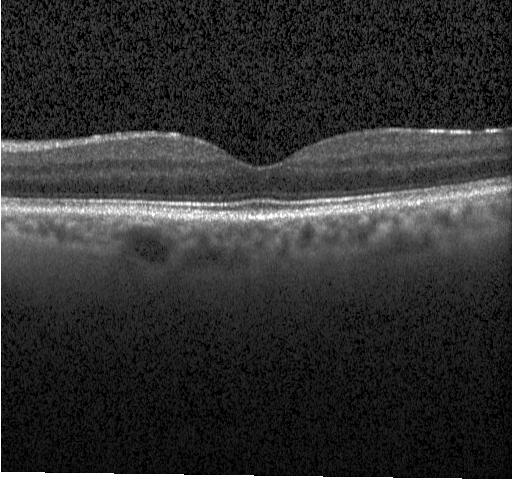

Impression: neither choroidal neovascularization, diabetic macular edema, nor drusen.